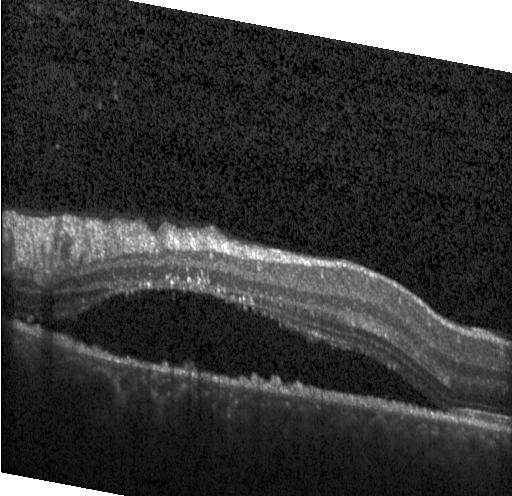 Finding: a choroidal neovascular membrane.